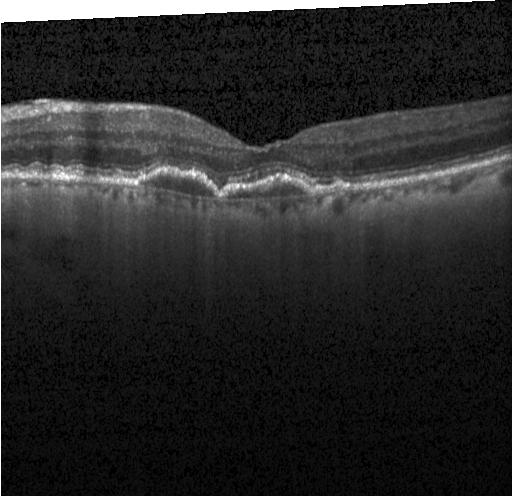
Retinal OCT cross-section. Diagnosis: choroidal neovascularization (CNV).